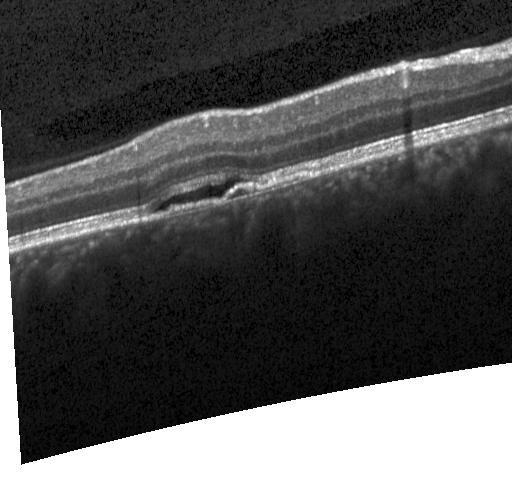

Fovea-centered, spectral-domain optical coherence tomography, retinal OCT cross-section, instrument: Heidelberg Spectralis. Finding: CNV.